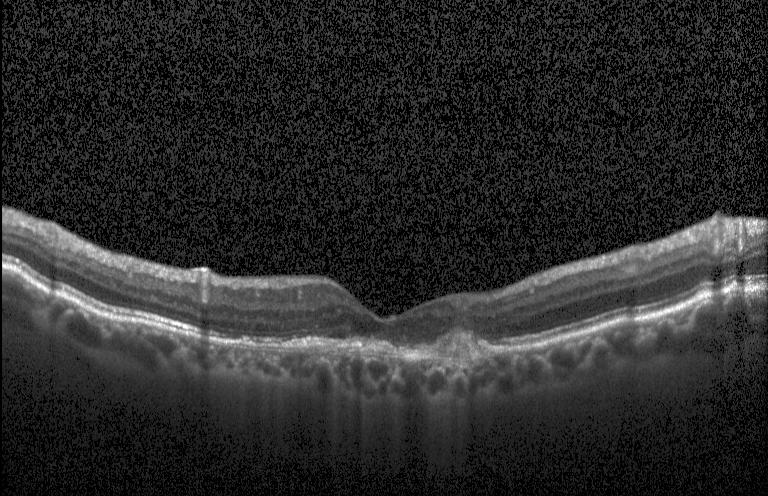
Finding: choroidal neovascularization.